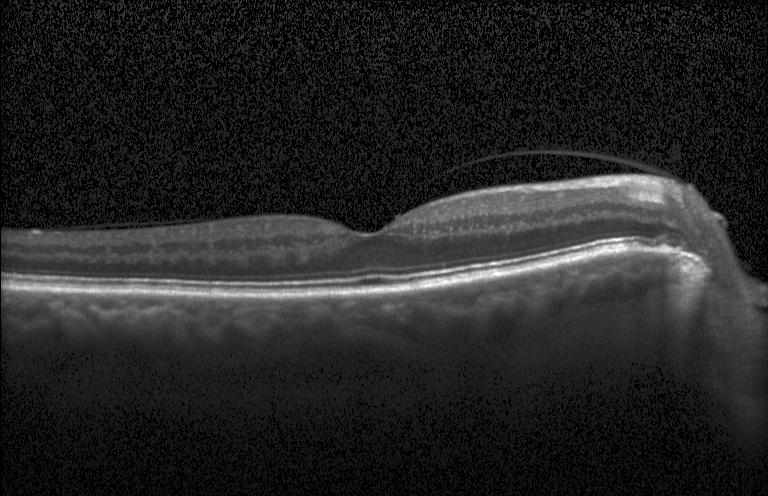 SD-OCT, optical coherence tomography scan.
Diagnosis: neither choroidal neovascularization, diabetic macular edema, nor drusen.